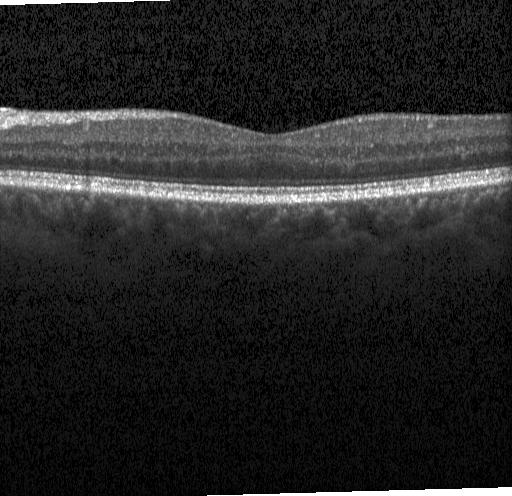
OCT B-scan showing neither choroidal neovascularization, diabetic macular edema, nor drusen.